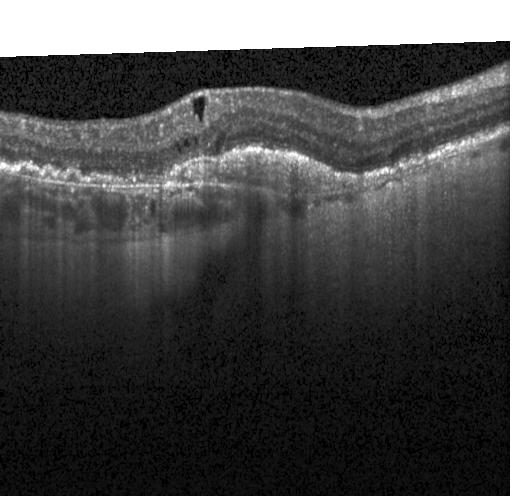
Impression: CNV.